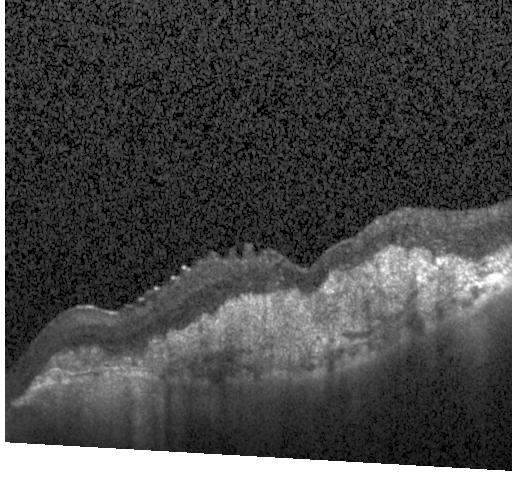
OCT line scan
Assessment: a choroidal neovascular membrane.